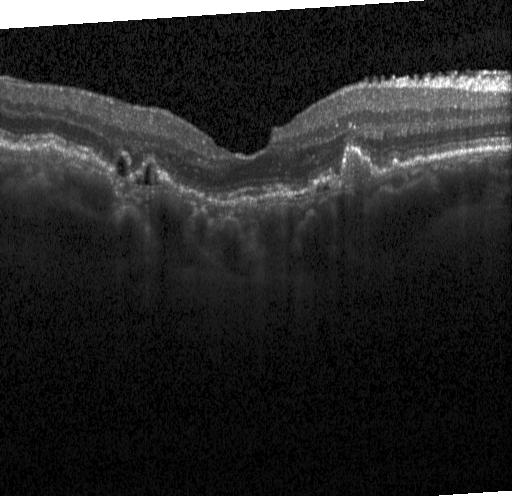 Spectral-domain optical coherence tomography; acquired on a Heidelberg Spectralis; OCT B-scan.
This B-scan demonstrates a choroidal neovascular membrane.